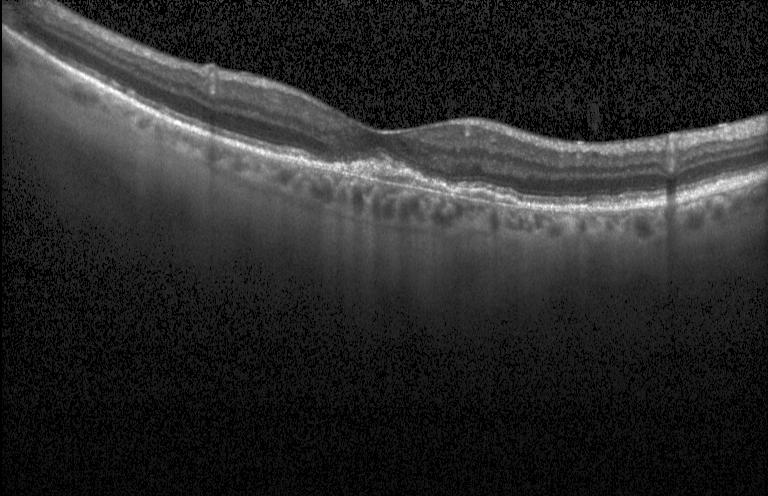 Spectral-domain OCT; Heidelberg Spectralis OCT system; retinal OCT B-scan.
Impression: choroidal neovascularization.